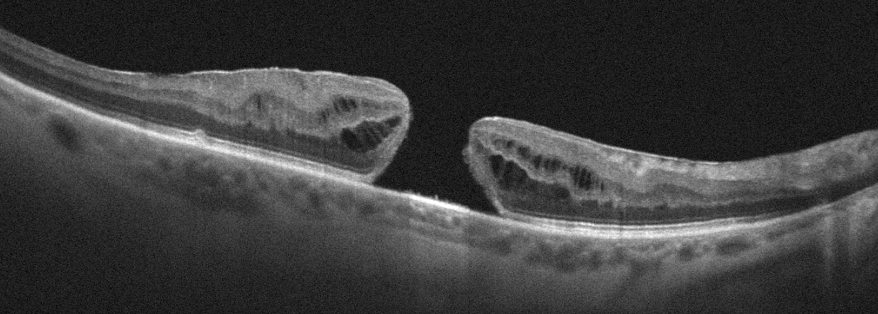 Macular OCT: vitreomacular interface disease.